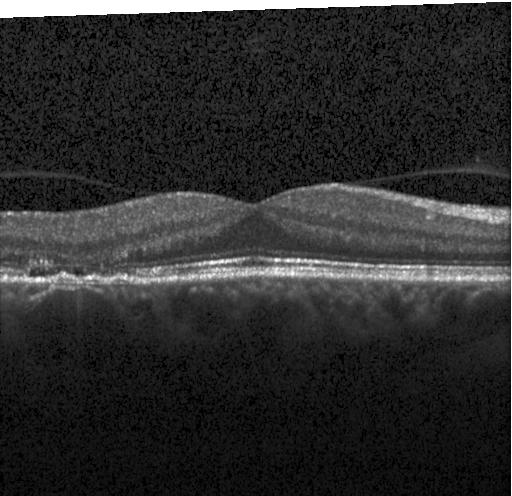 Optical coherence tomography scan. SD-OCT
Finding: a choroidal neovascular membrane.